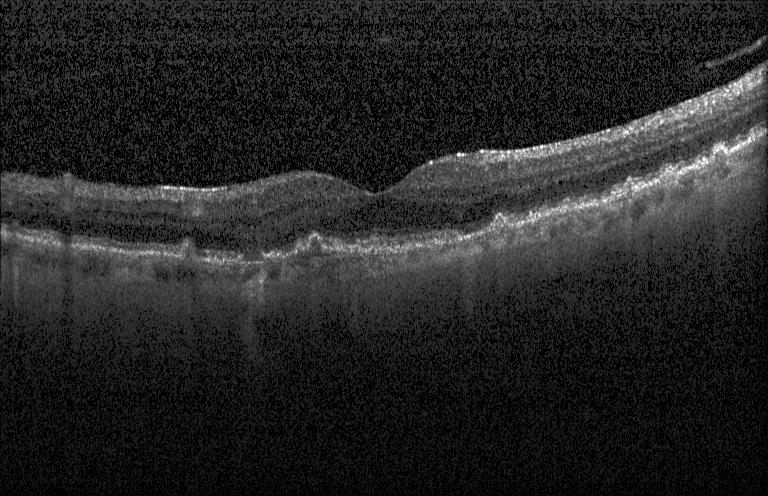

Optical coherence tomography scan. Impression: sub-RPE drusenoid deposits.